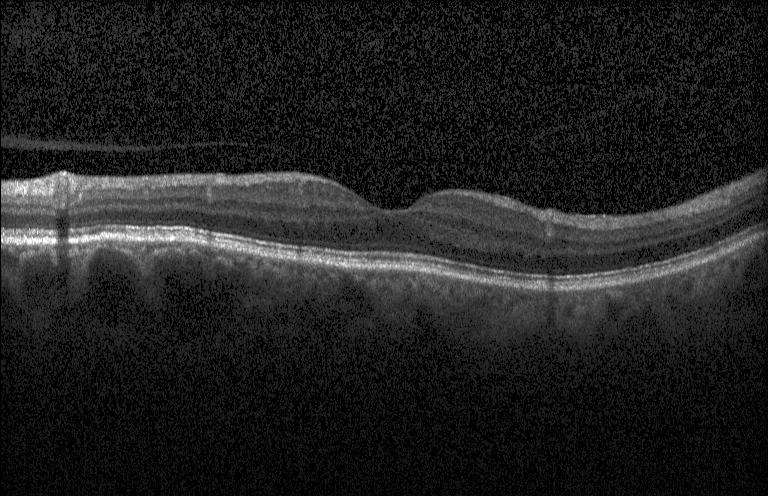 SD-OCT. Horizontal scan through the fovea. OCT B-scan — No evidence of choroidal neovascularization, diabetic macular edema, or drusen.